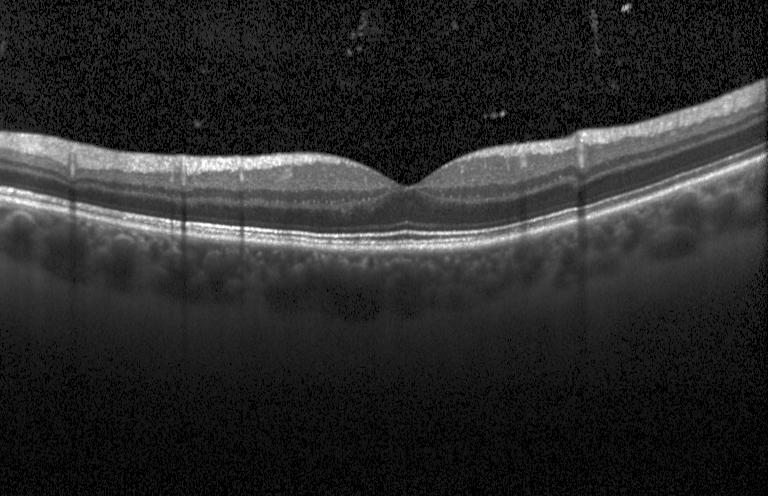 Macular scan; spectral-domain optical coherence tomography; retinal OCT B-scan
Finding: no CNV, no DME, and no drusen.